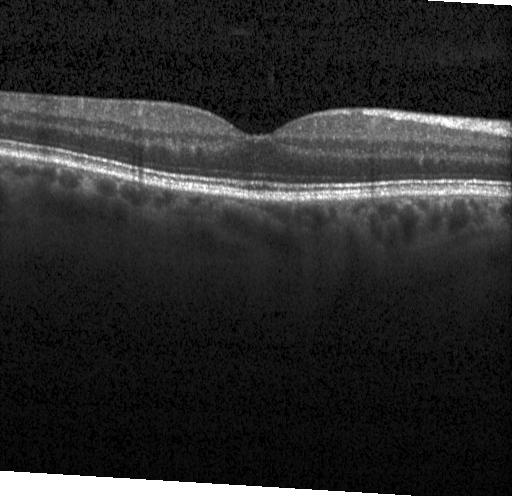 Finding: no choroidal neovascularization, diabetic macular edema, or drusen.